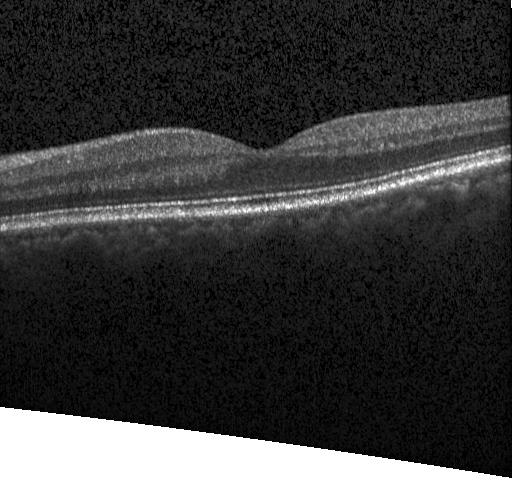
Fovea-centered · retinal OCT cross-section
Assessment: no choroidal neovascularization, no diabetic macular edema, and no drusen.